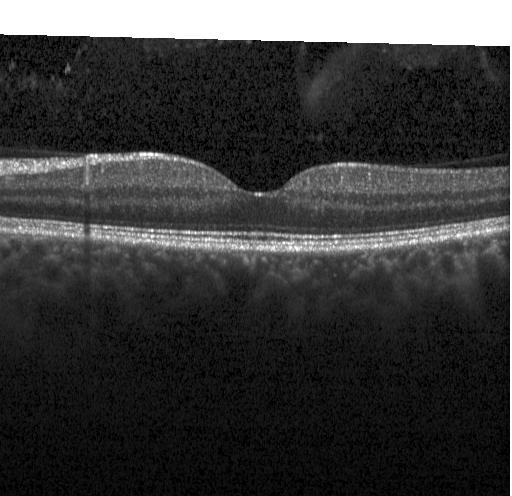

Retinal OCT B-scan
No choroidal neovascularization, no diabetic macular edema, and no drusen.